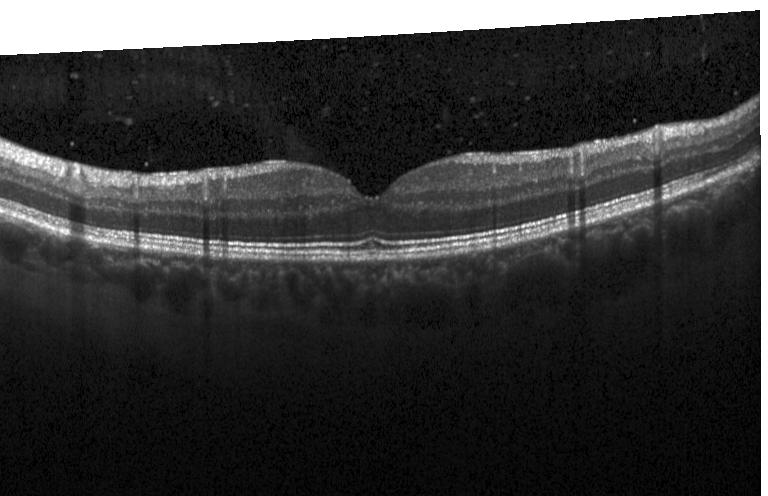 SD-OCT. Macular scan. Heidelberg Spectralis. OCT line scan — OCT finding: no evidence of CNV, DME, or drusen.